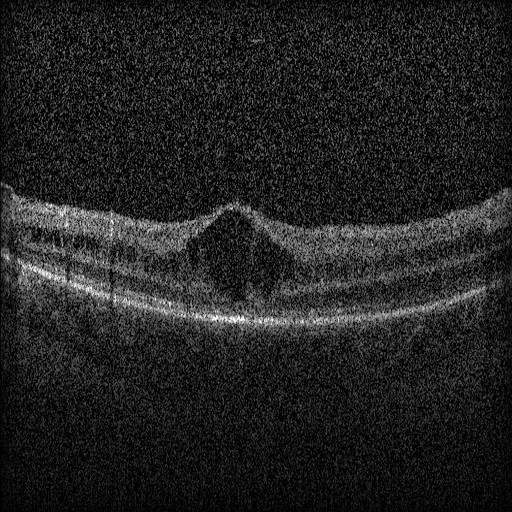 Optical coherence tomography scan
Impression: DME.